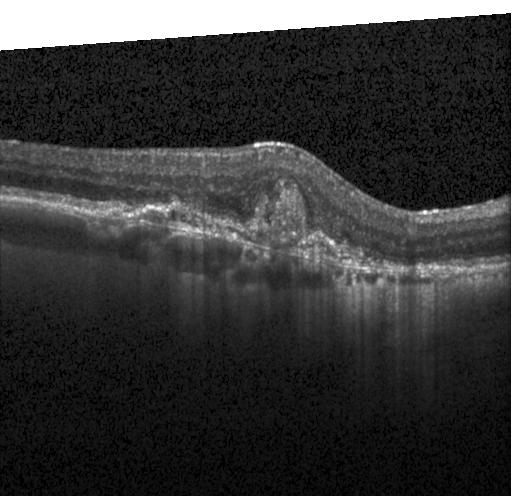 OCT line scan.
The scan shows a choroidal neovascular membrane.